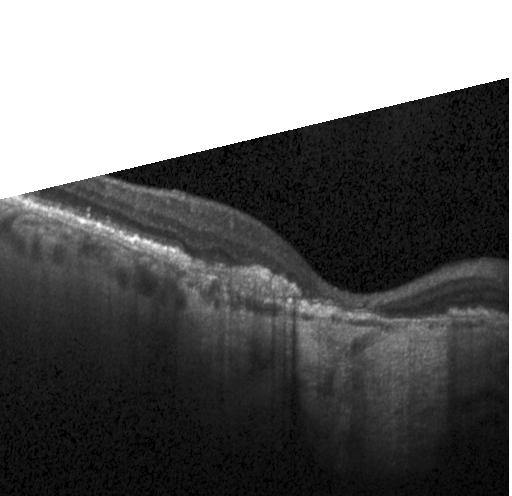 Impression: CNV.